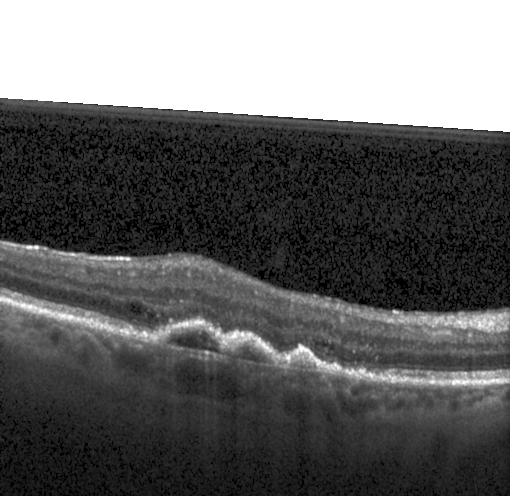
OCT line scan.
This B-scan demonstrates choroidal neovascularization (CNV).